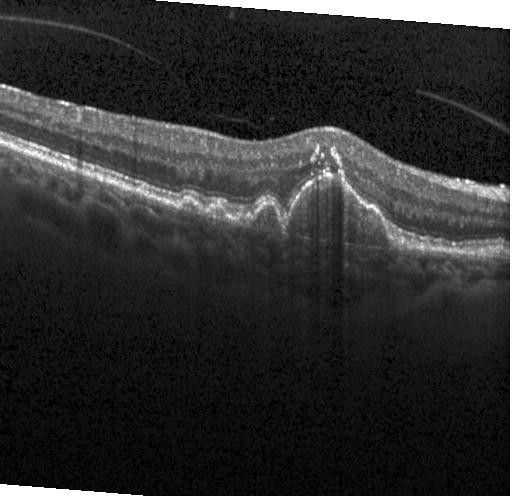
Diagnosis: a choroidal neovascular membrane.